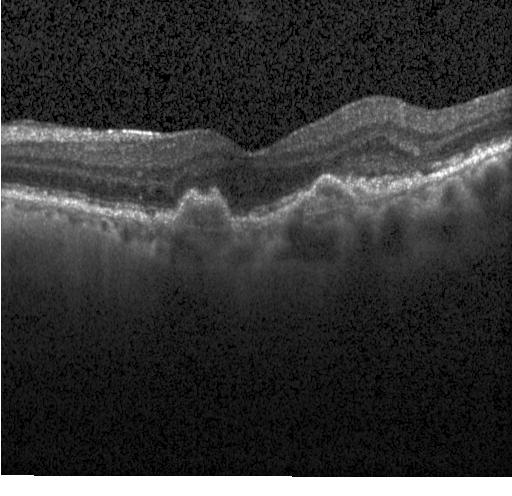 Retinal OCT cross-section showing choroidal neovascularization (CNV).